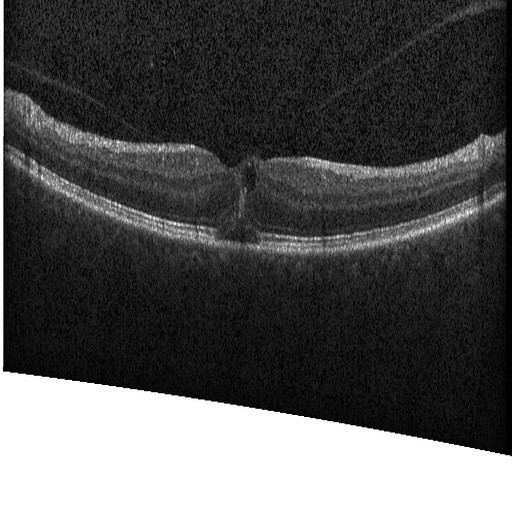 Optical coherence tomography scan · fovea-centered · Heidelberg Spectralis · spectral-domain OCT. Impression: diabetic macular edema.